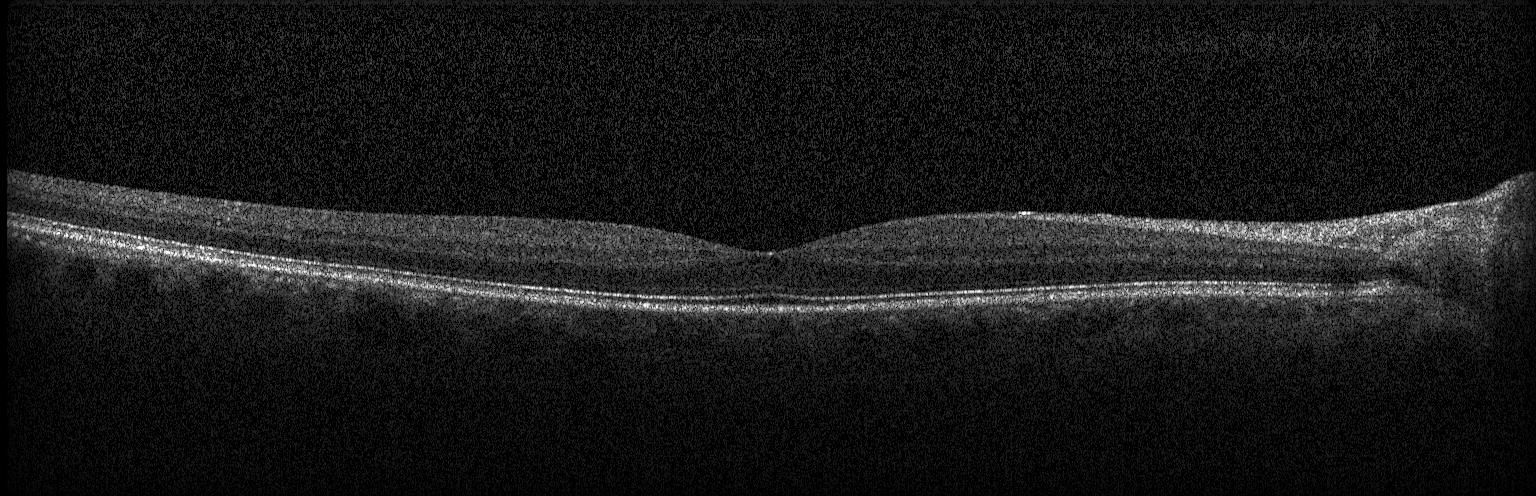 Heidelberg Spectralis · SD-OCT · OCT B-scan. Neither choroidal neovascularization, diabetic macular edema, nor drusen.